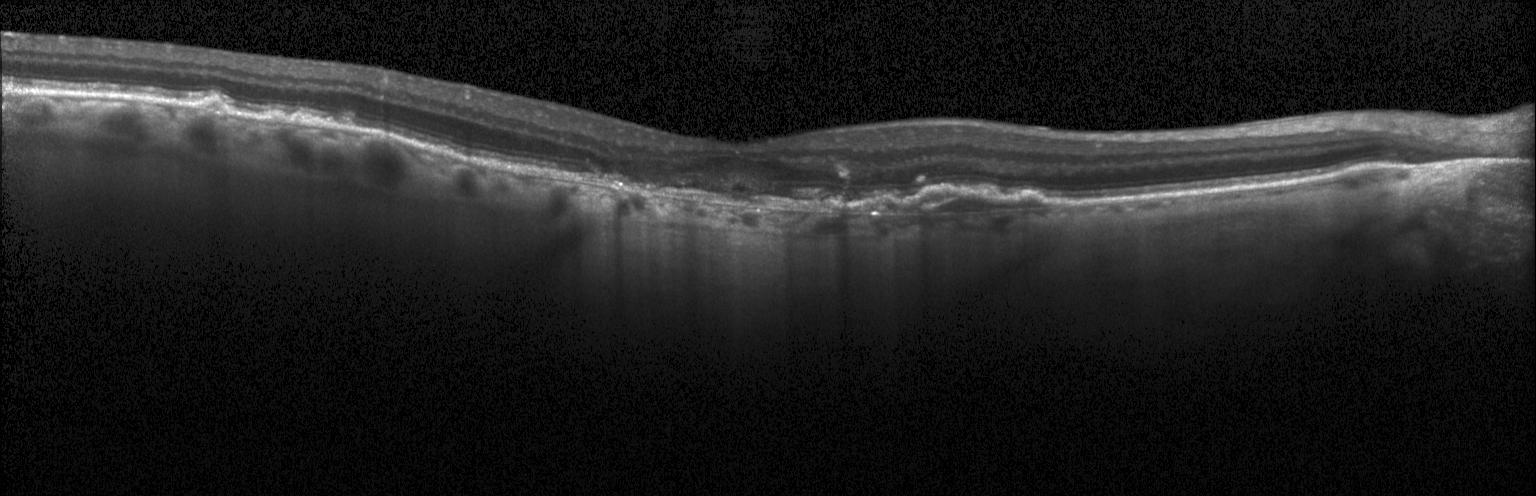 OCT line scan. The scan shows a choroidal neovascular membrane.